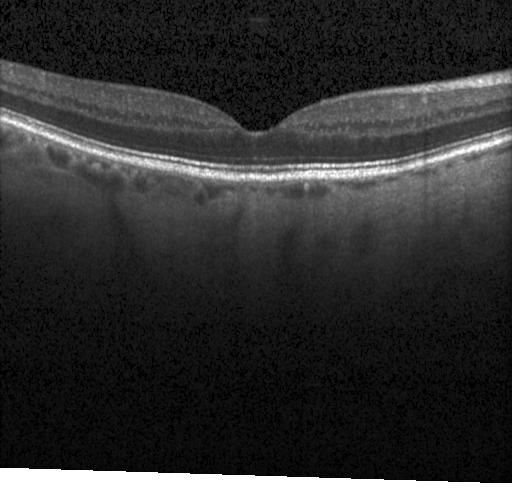
Spectral-domain OCT B-scan: neither CNV, DME, nor drusen.